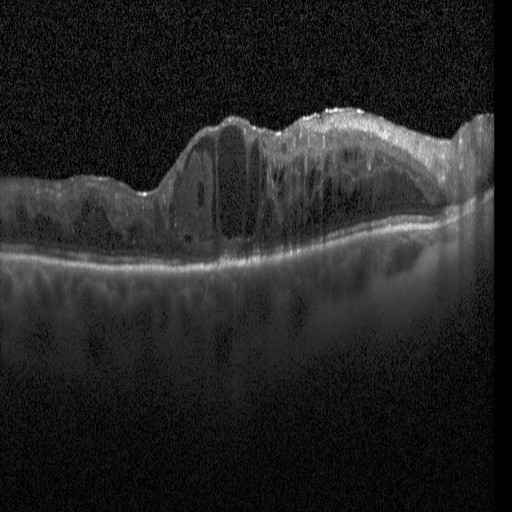

Heidelberg Spectralis. Retinal OCT cross-section. SD-OCT.
Macular OCT: diabetic macular edema.